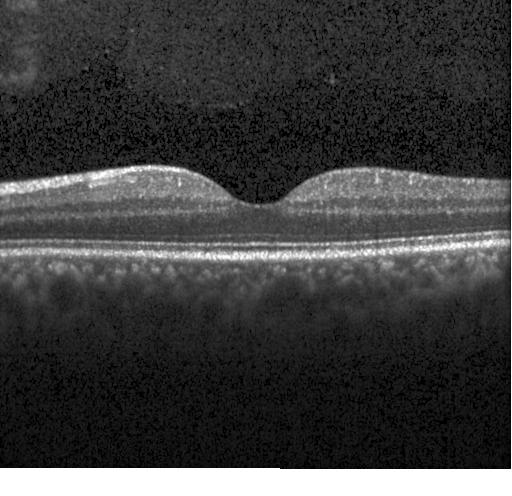

Spectral-domain optical coherence tomography. Heidelberg Spectralis OCT system. OCT B-scan — This B-scan demonstrates no evidence of CNV, DME, or drusen.